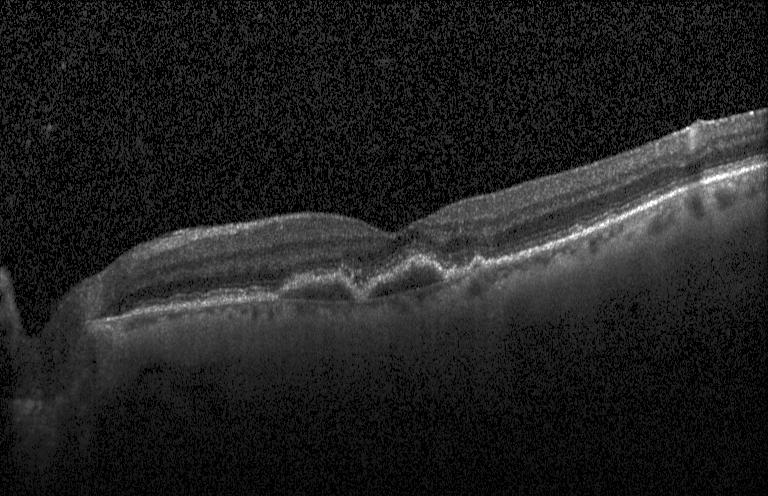 OCT B-scan. Acquired on a Heidelberg Spectralis. SD-OCT. Horizontal scan through the fovea — Dx: choroidal neovascularization (CNV).